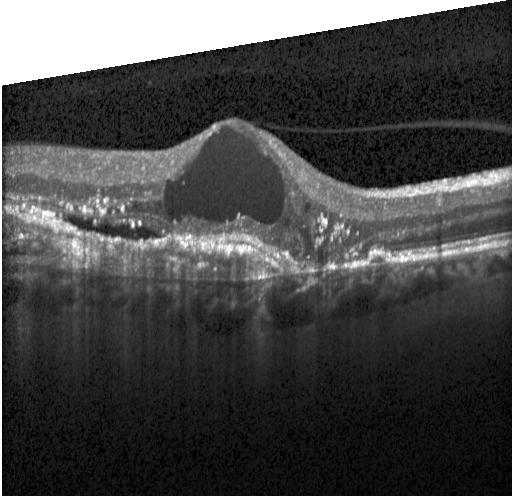 Spectral-domain OCT B-scan: choroidal neovascularization.